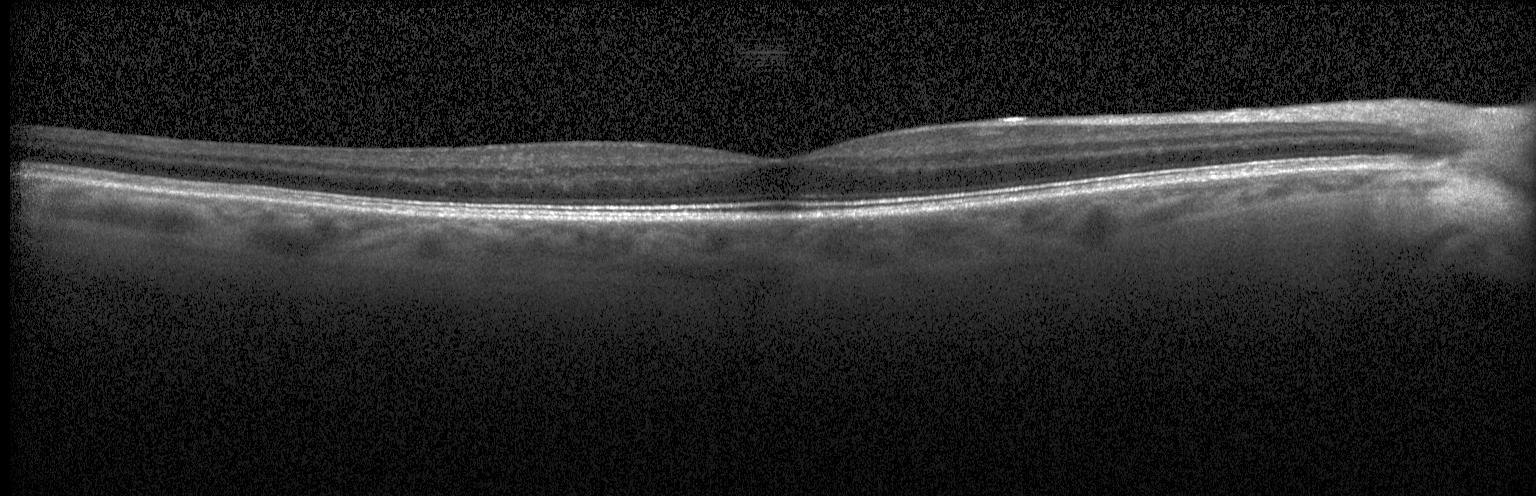

Diagnosis: no evidence of CNV, DME, or drusen.